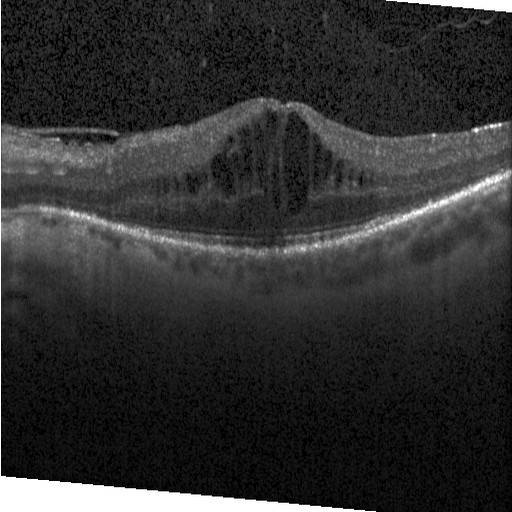
Optical coherence tomography scan, SD-OCT, macular scan, acquired on a Heidelberg Spectralis
Macular OCT: DME.